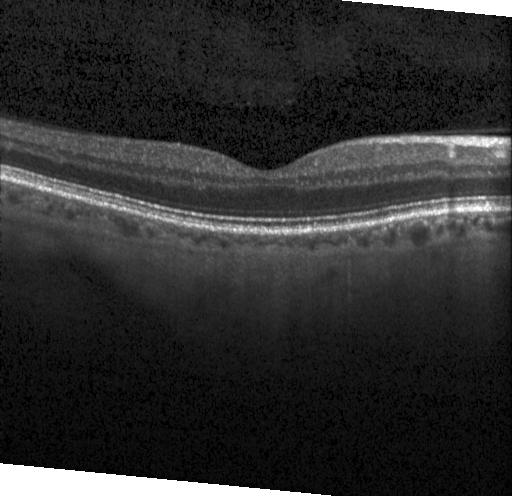

OCT B-scan — Diagnosis: no choroidal neovascularization, no diabetic macular edema, and no drusen.